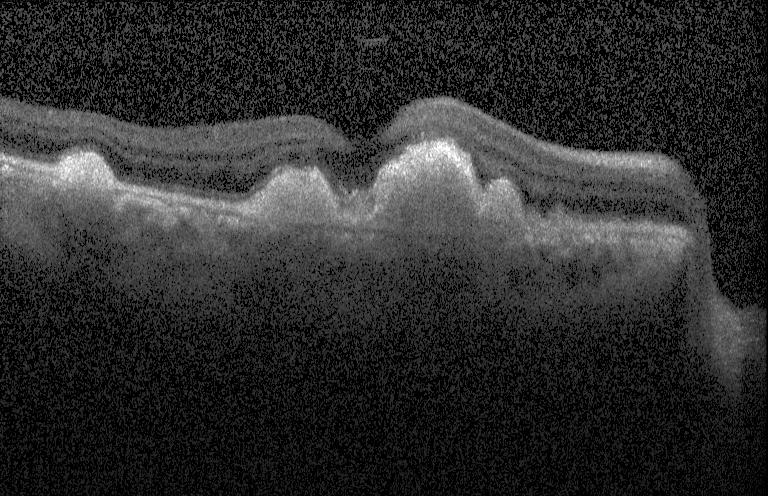
Retinal OCT B-scan. Instrument: Heidelberg Spectralis — Diagnosis: drusen.